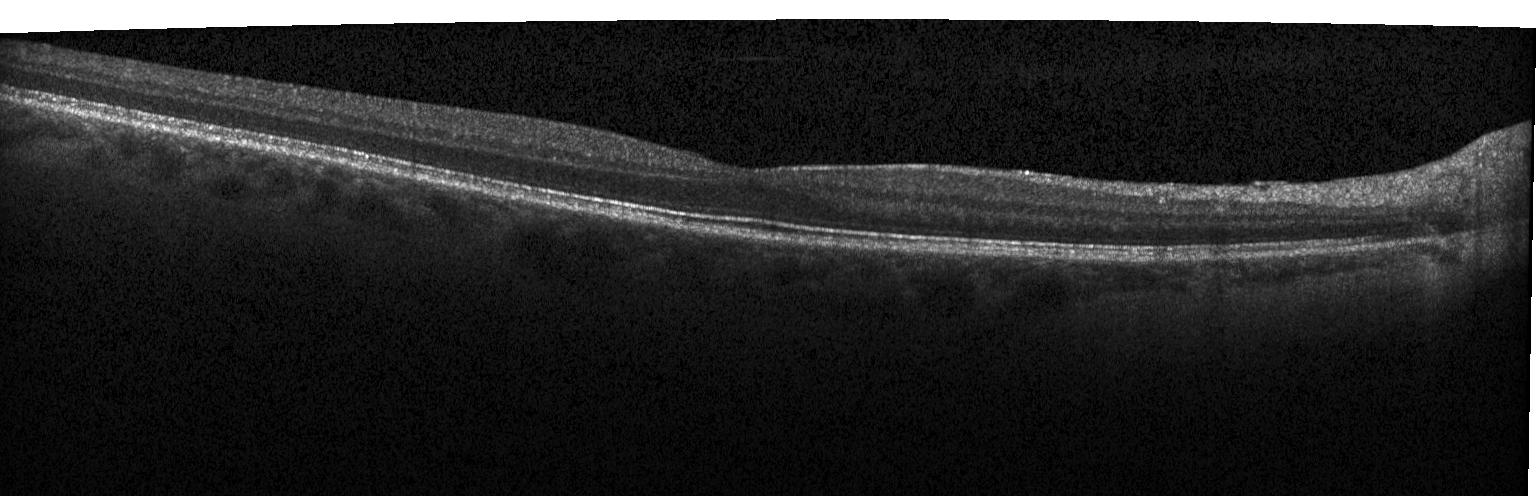

This B-scan demonstrates no choroidal neovascularization, diabetic macular edema, or drusen.